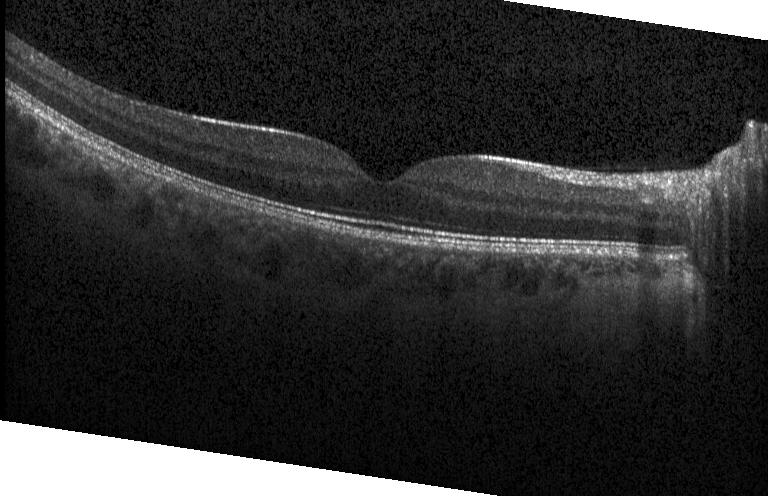

Macular OCT: no choroidal neovascularization, diabetic macular edema, or drusen.